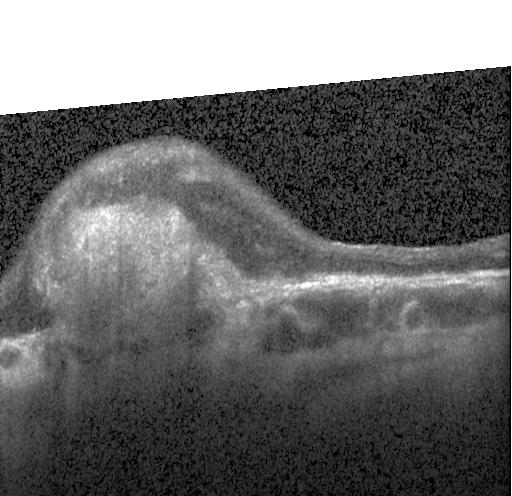
SD-OCT. Heidelberg Spectralis OCT system. Centered on the fovea. OCT B-scan — Finding: a choroidal neovascular membrane.